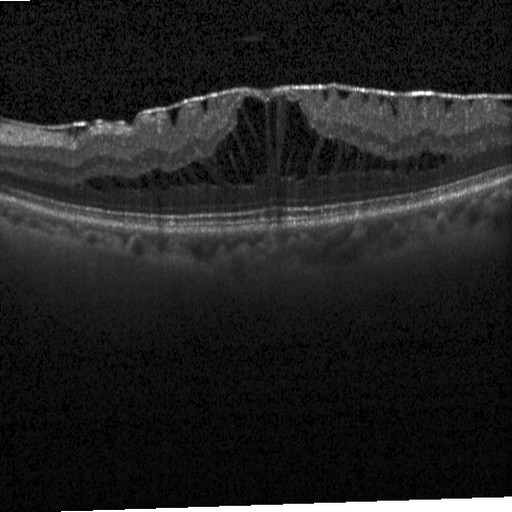
Retinal OCT B-scan.
Diabetic macular edema (DME).